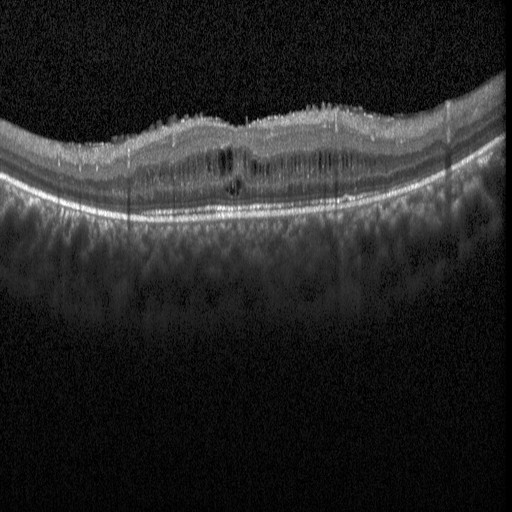
Impression: DME.